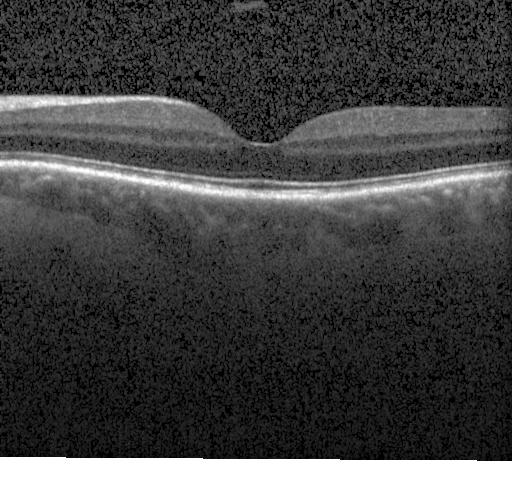
Spectral-domain optical coherence tomography, OCT B-scan, instrument: Heidelberg Spectralis — Dx: neither CNV, DME, nor drusen.